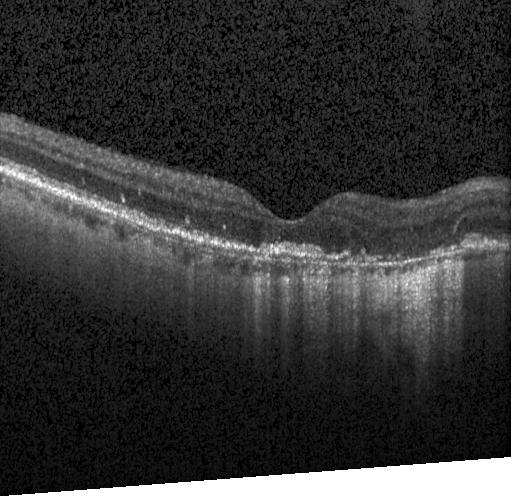
Optical coherence tomography B-scan — Dx: a choroidal neovascular membrane.